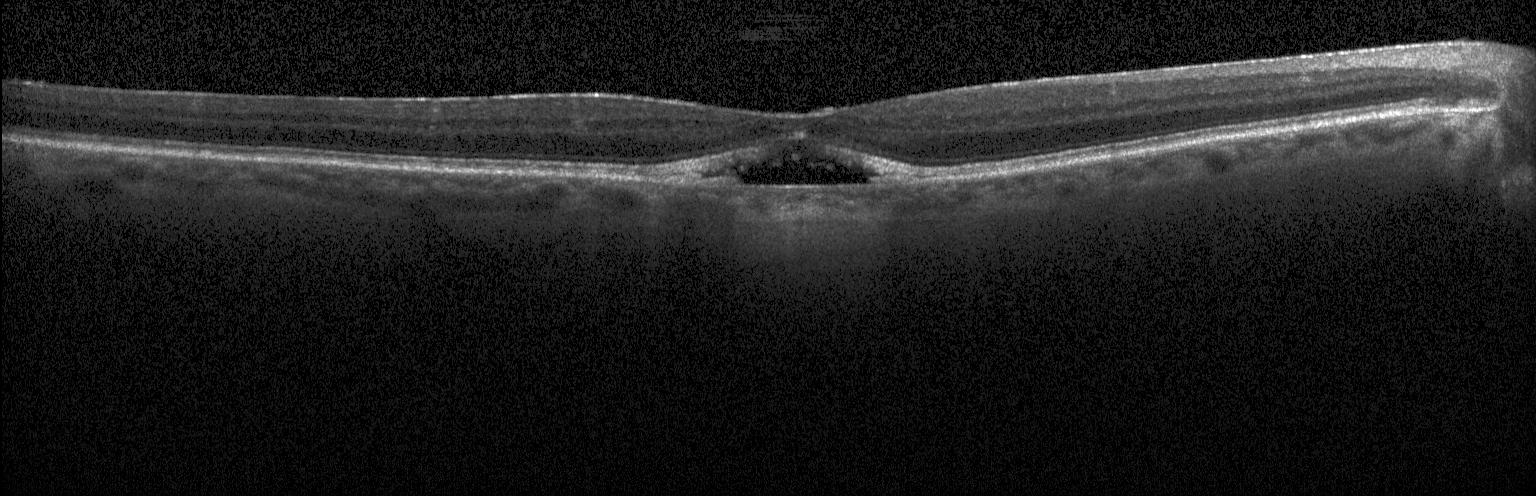

Diagnosis: CNV.